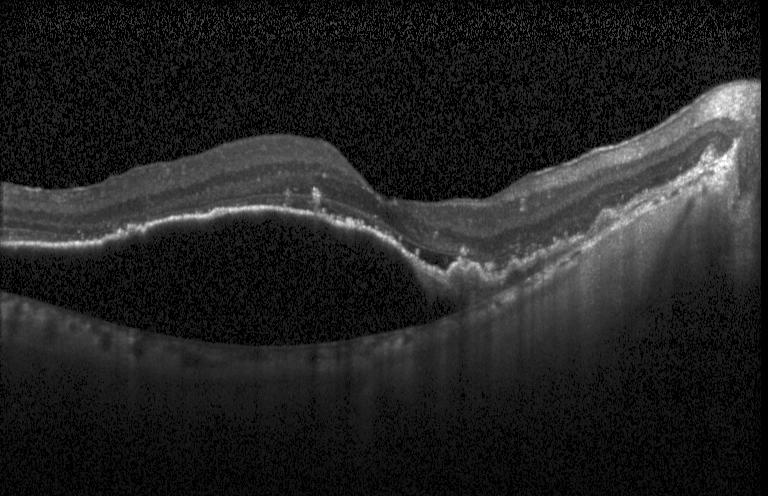 The scan shows CNV.